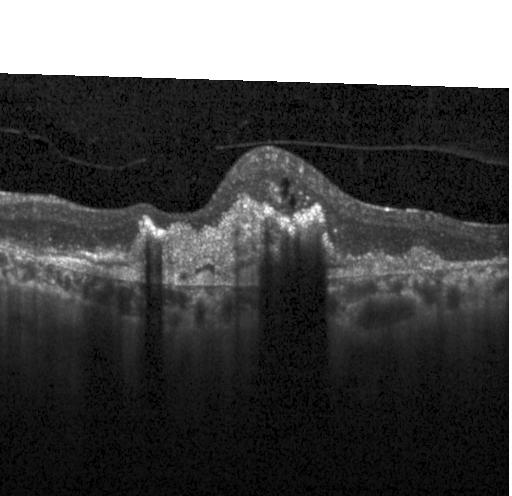

Spectral-domain OCT · OCT line scan · Heidelberg Spectralis
The scan shows a choroidal neovascular membrane.